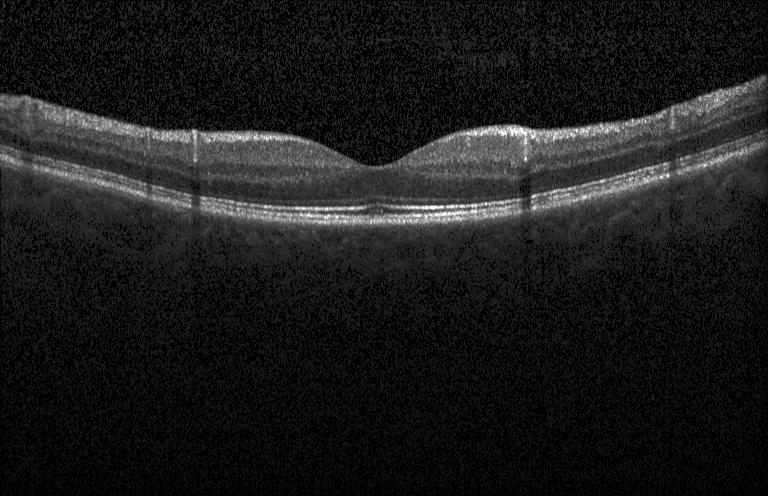
Retinal OCT cross-section. SD-OCT.
OCT finding: no choroidal neovascularization, no diabetic macular edema, and no drusen.